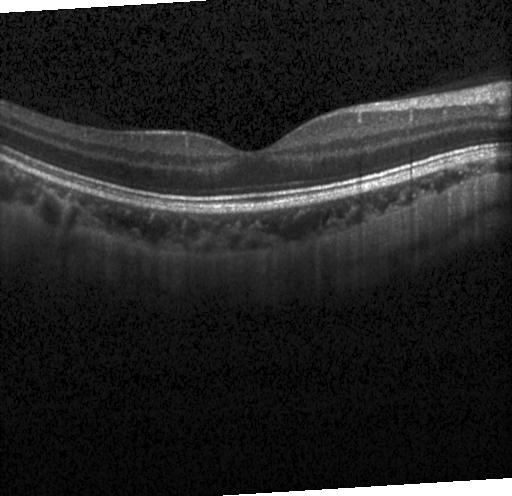

Retinal OCT cross-section.
Assessment: neither CNV, DME, nor drusen.